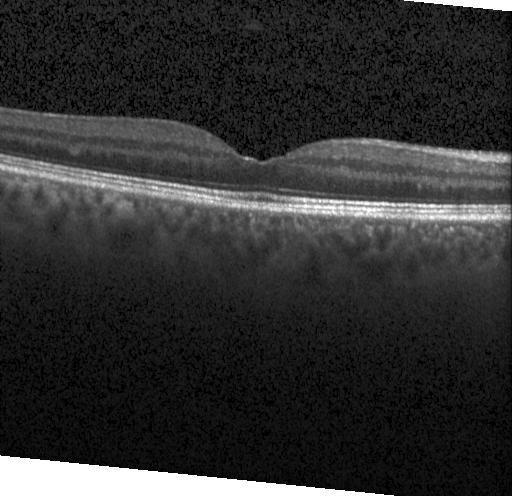
OCT B-scan. Impression: no CNV, no DME, and no drusen.